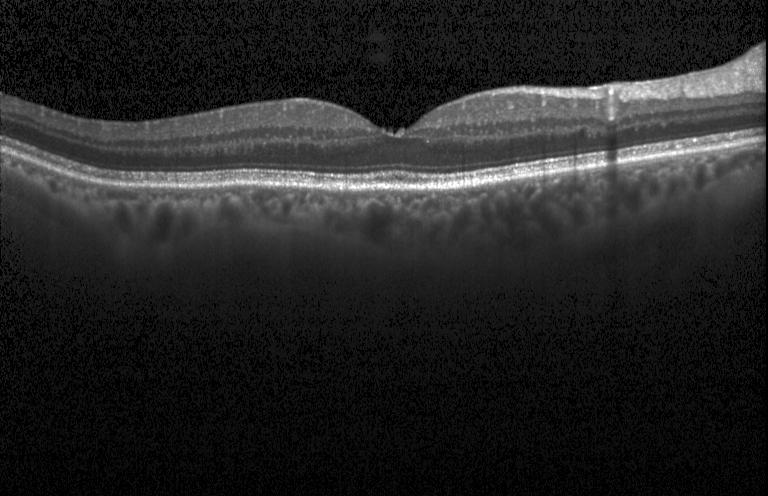
Retinal OCT B-scan — Finding: no choroidal neovascularization, diabetic macular edema, or drusen.